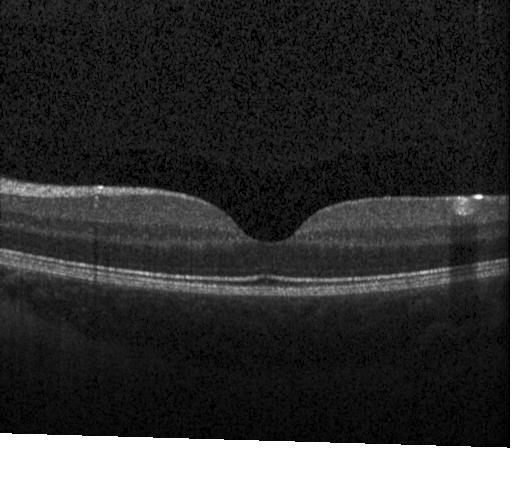
OCT B-scan showing no choroidal neovascularization, diabetic macular edema, or drusen.